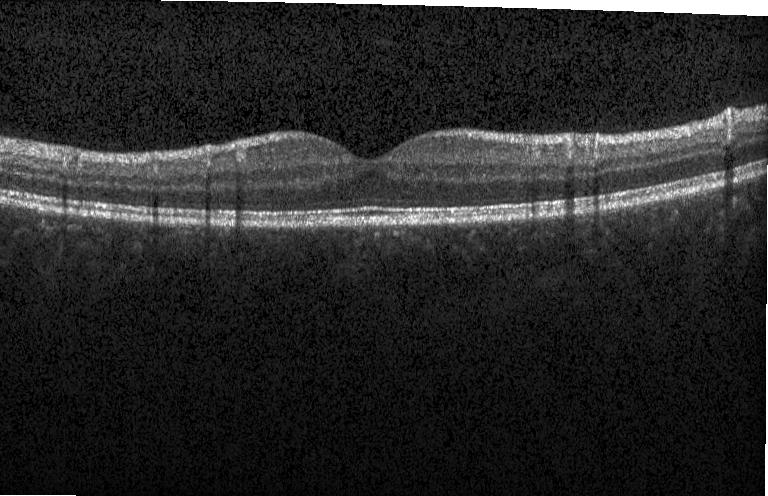

Retinal OCT cross-section showing no evidence of choroidal neovascularization, diabetic macular edema, or drusen.